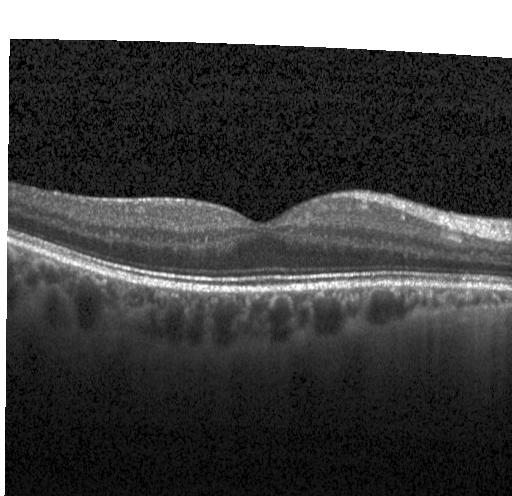 Optical coherence tomography B-scan. Acquired on a Heidelberg Spectralis. Finding: no CNV, DME, or drusen.